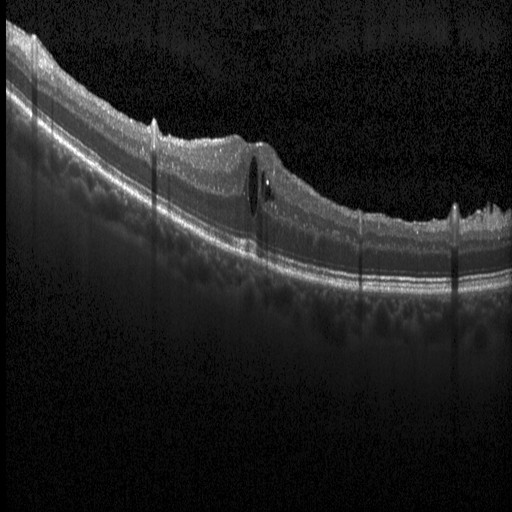
OCT line scan — The scan shows diabetic macular edema (DME).